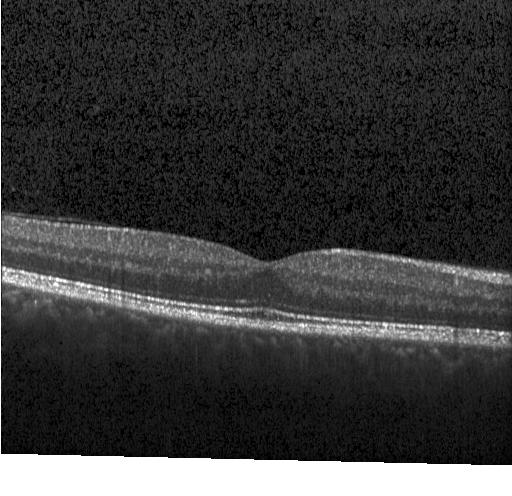

Heidelberg Spectralis, optical coherence tomography scan, fovea-centered
Finding: no evidence of choroidal neovascularization, diabetic macular edema, or drusen.